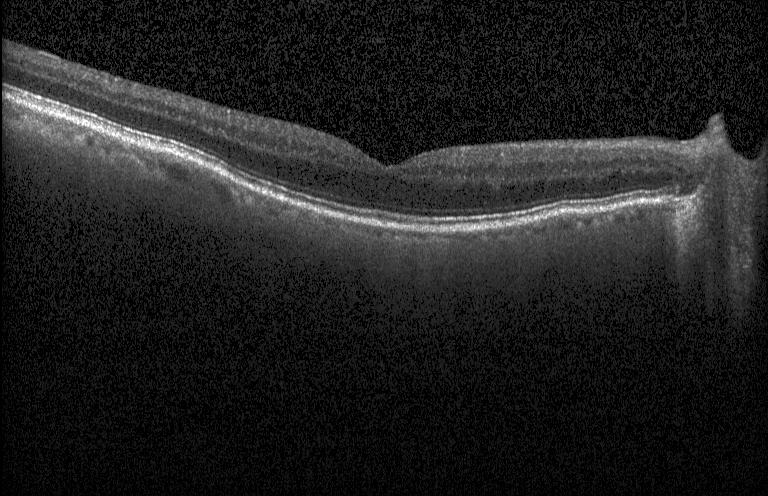

This B-scan demonstrates no choroidal neovascularization, no diabetic macular edema, and no drusen.